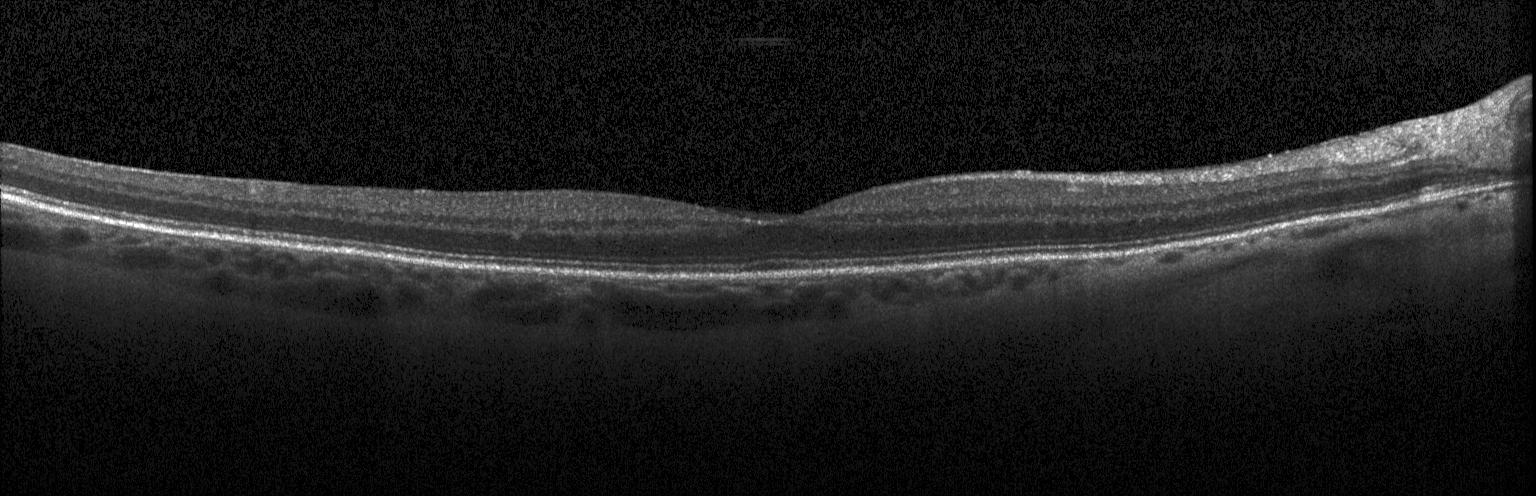
OCT B-scan; spectral-domain OCT
Diagnosis: no CNV, no DME, and no drusen.